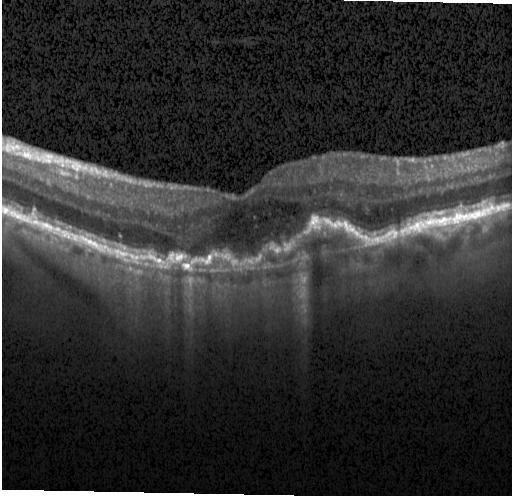 Horizontal scan through the fovea; retinal OCT cross-section. Diagnosis: a choroidal neovascular membrane.